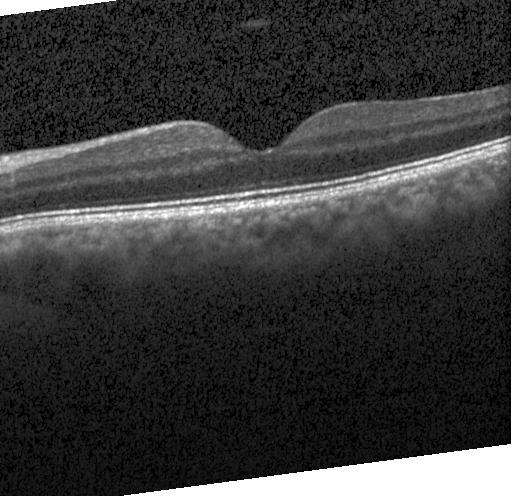
Heidelberg Spectralis. Horizontal scan through the fovea. OCT B-scan. Assessment: no CNV, DME, or drusen.